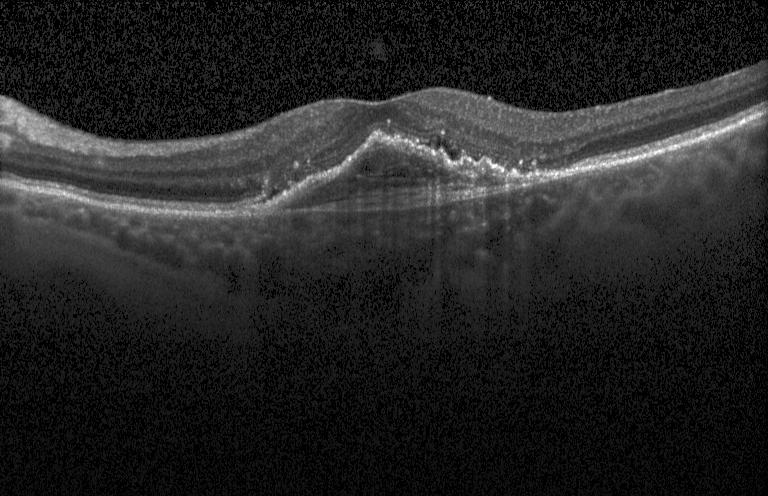

Heidelberg Spectralis, OCT line scan, through the macula
CNV.